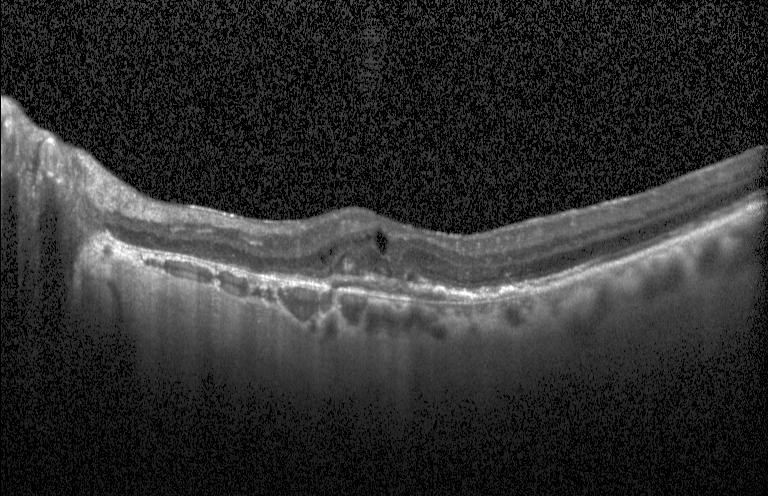 Macular OCT: choroidal neovascularization (CNV).